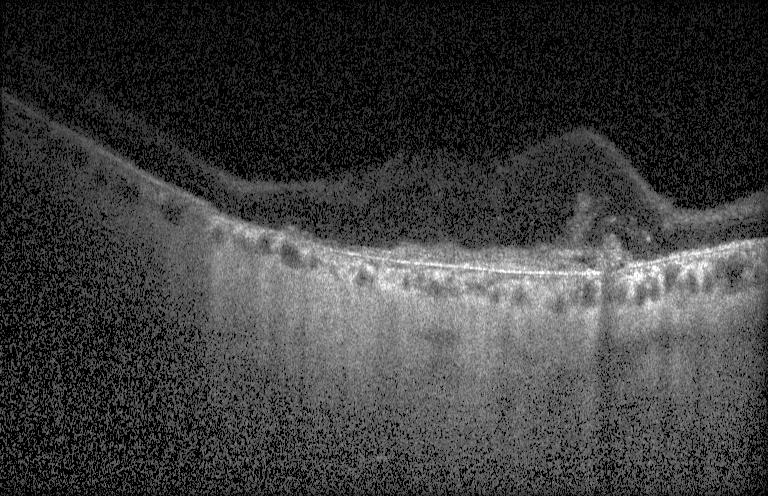 Choroidal neovascularization.